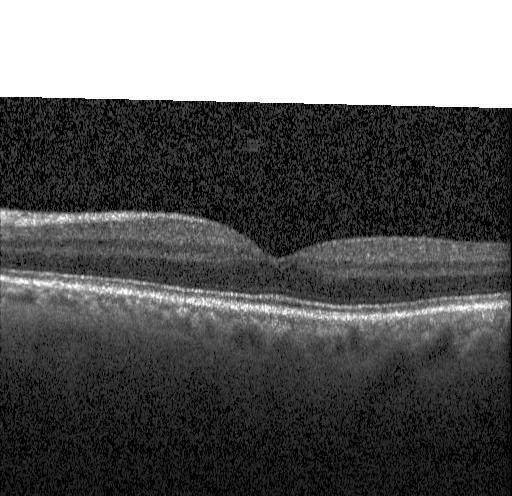

Finding: no CNV, no DME, and no drusen.